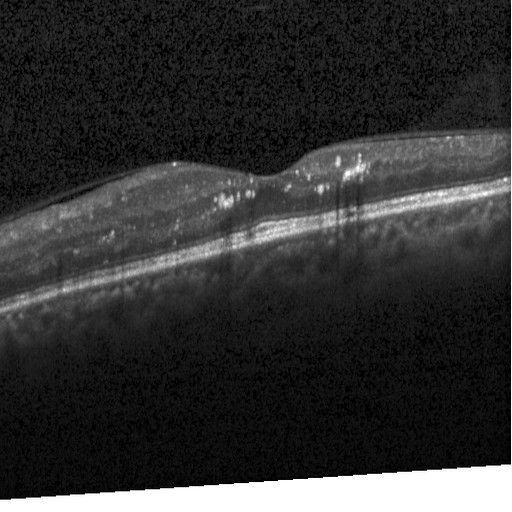
Diagnosis: DME.